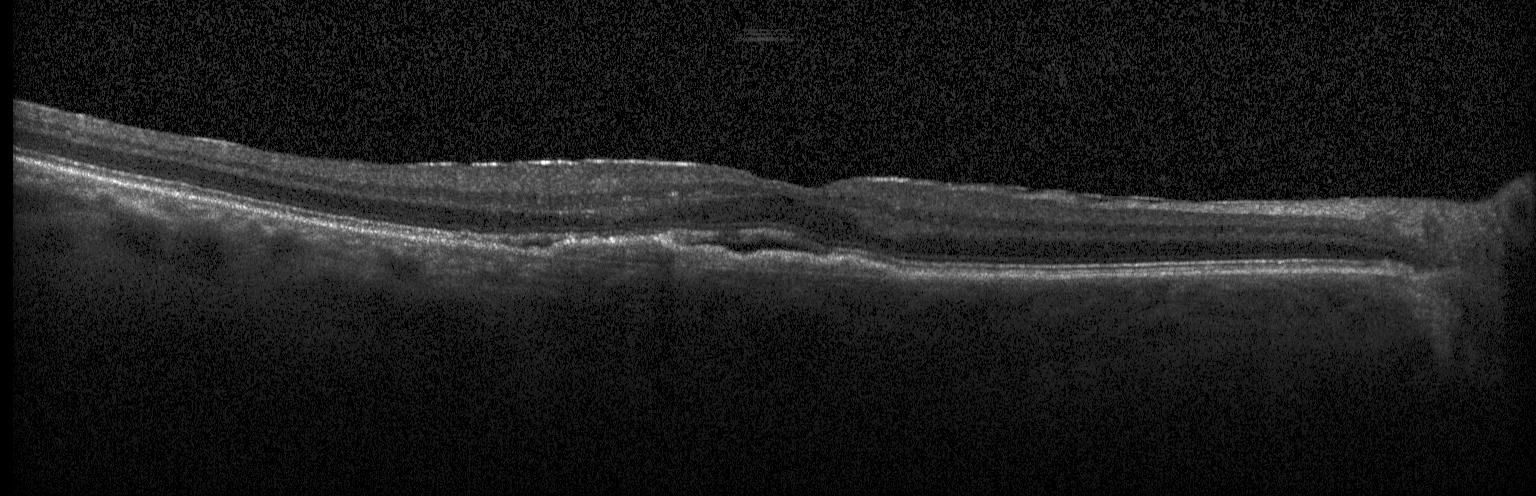
Optical coherence tomography B-scan; Heidelberg Spectralis OCT system; macular scan; spectral-domain optical coherence tomography.
A choroidal neovascular membrane.